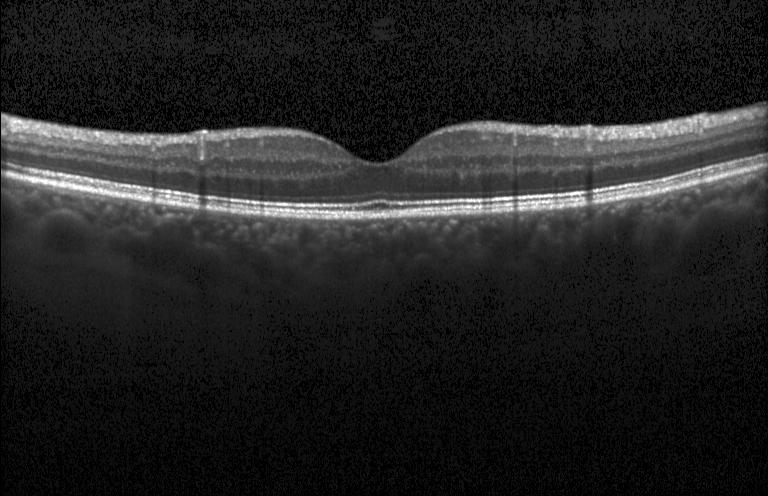
Retinal OCT cross-section · horizontal scan through the fovea · instrument: Heidelberg Spectralis. Diagnosis: no choroidal neovascularization, no diabetic macular edema, and no drusen.